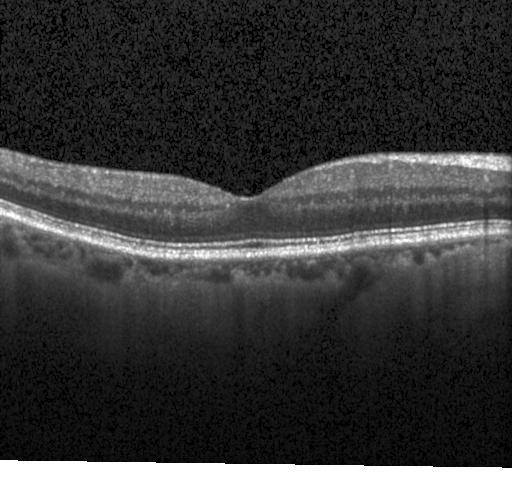 Acquired on a Heidelberg Spectralis. OCT line scan. Fovea-centered
This B-scan demonstrates no choroidal neovascularization, no diabetic macular edema, and no drusen.